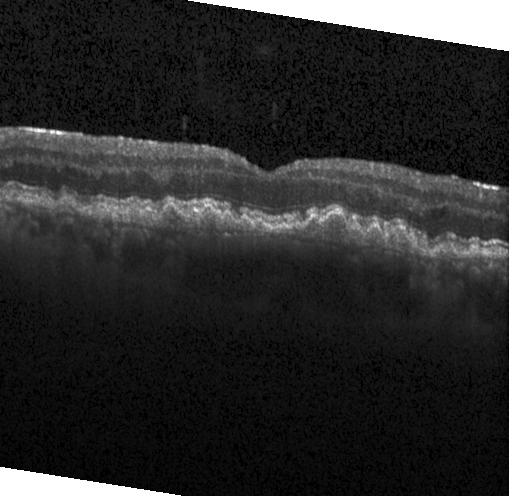 Heidelberg Spectralis OCT system; spectral-domain optical coherence tomography; fovea-centered; retinal OCT B-scan
Finding: a choroidal neovascular membrane.